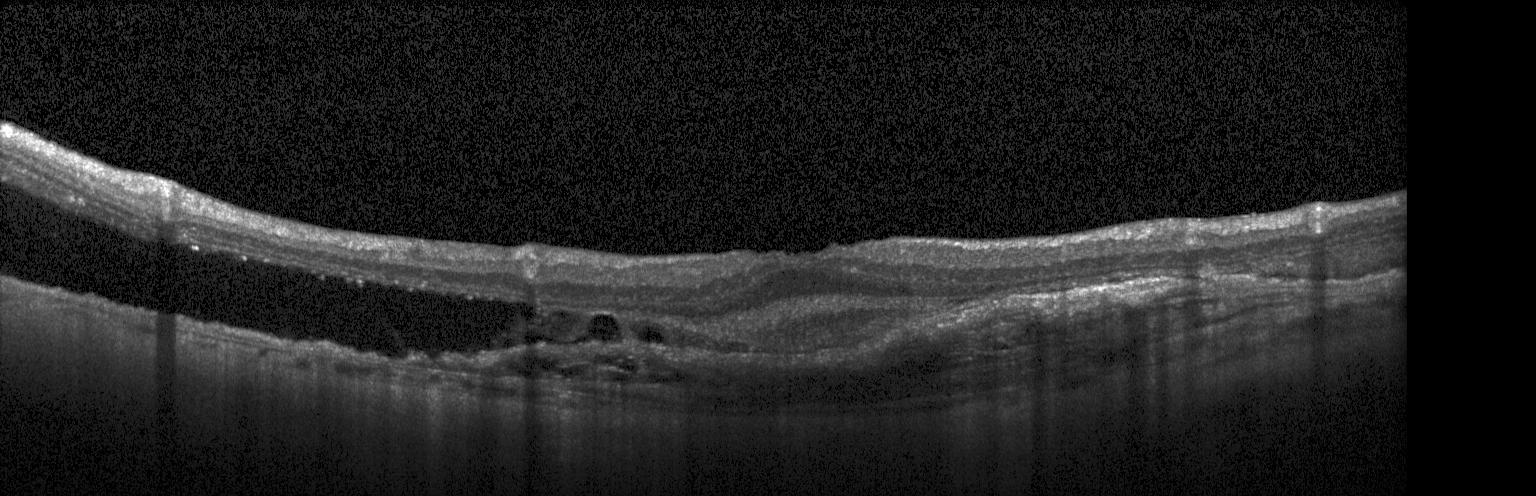
Retinal OCT B-scan. Diagnosis: a choroidal neovascular membrane.